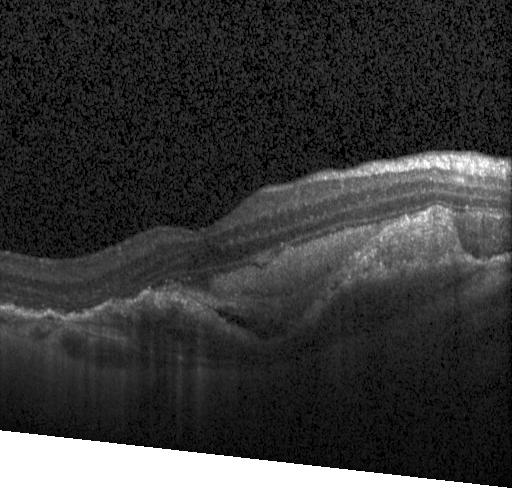

OCT line scan — The scan shows a choroidal neovascular membrane.